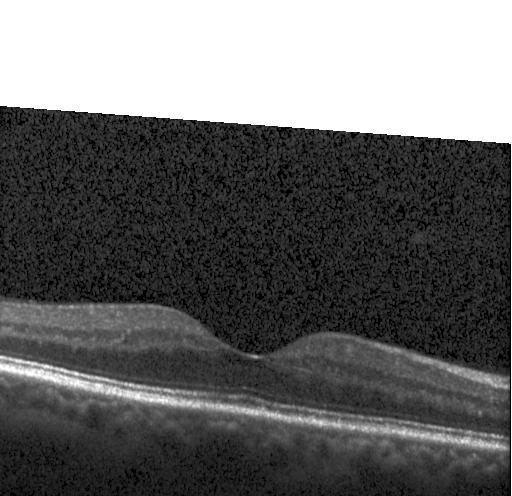
This B-scan demonstrates no choroidal neovascularization, no diabetic macular edema, and no drusen.